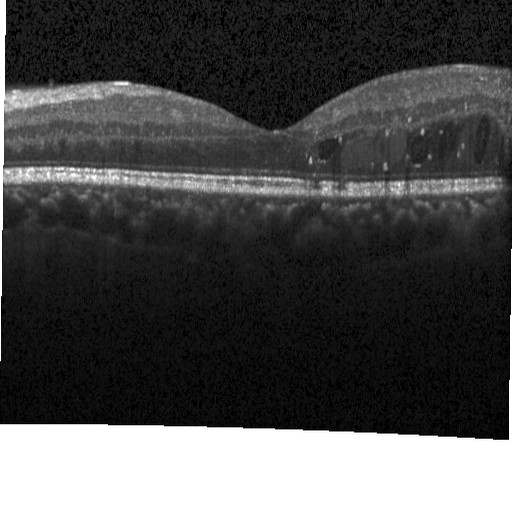

Retinal OCT B-scan. This B-scan demonstrates diabetic macular edema (DME).